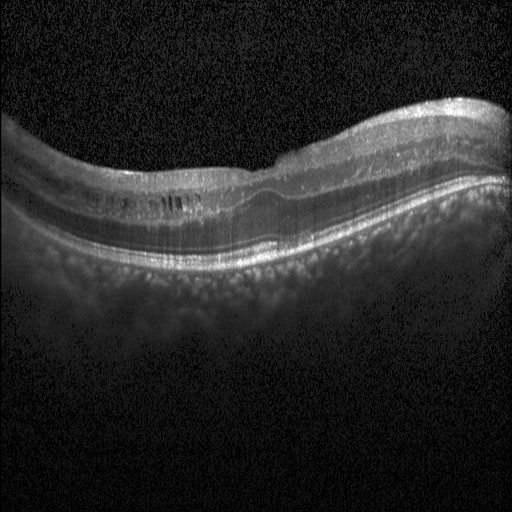

SD-OCT, Heidelberg Spectralis OCT system, retinal OCT B-scan. Impression: diabetic macular edema (DME).